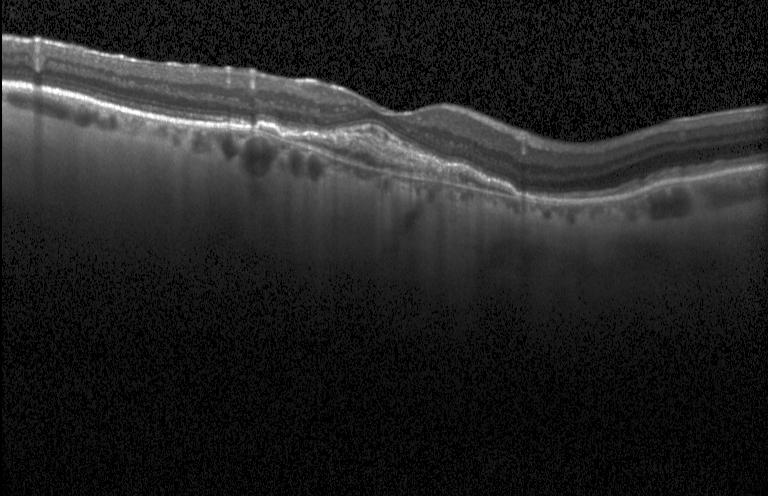

OCT B-scan showing a choroidal neovascular membrane.